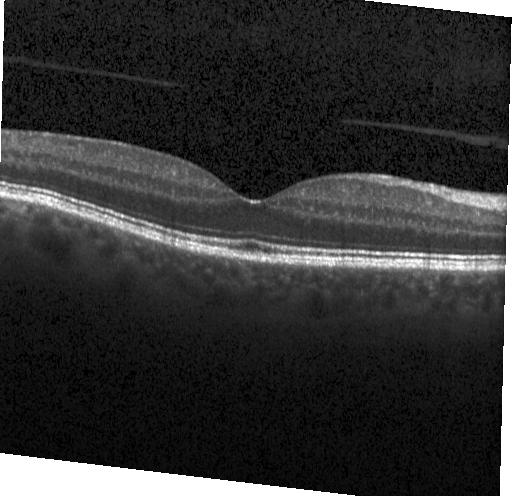
Spectral-domain OCT B-scan: neither choroidal neovascularization, diabetic macular edema, nor drusen.